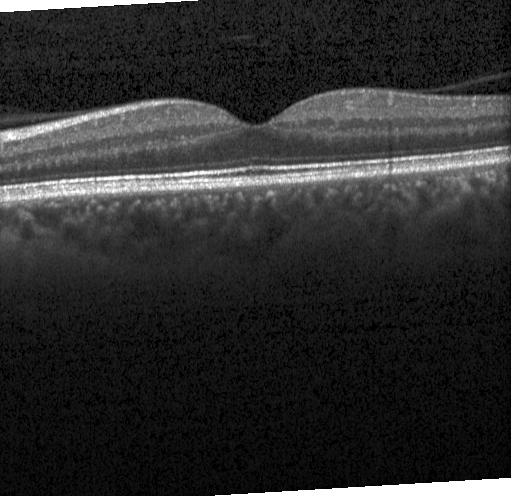 OCT B-scan — Finding: neither CNV, DME, nor drusen.